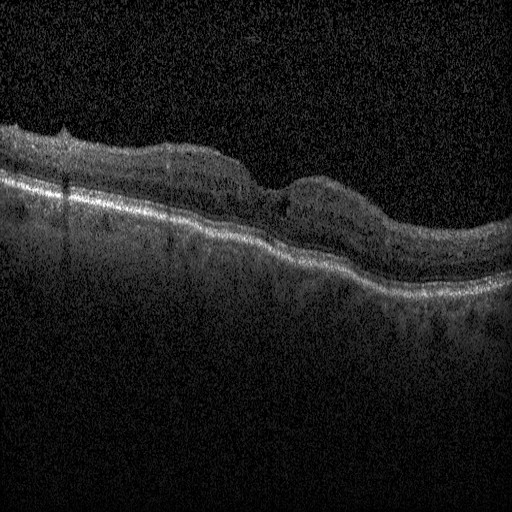 Retinal OCT B-scan, through the macula, Heidelberg Spectralis, SD-OCT.
Diagnosis: diabetic macular edema (DME).